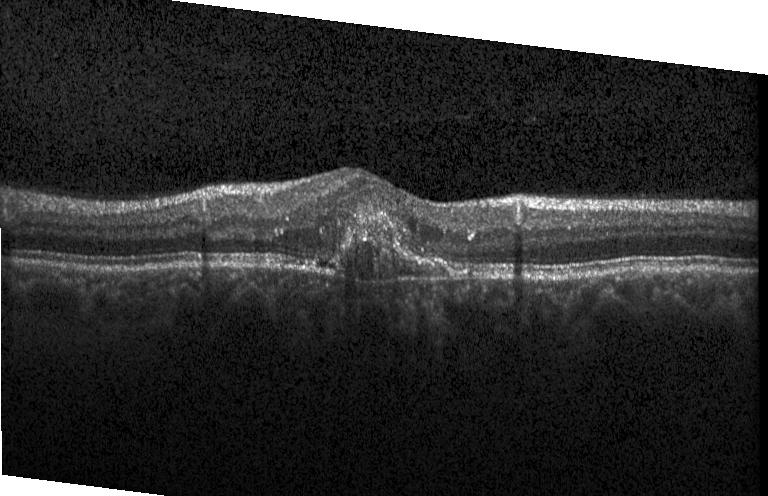

Assessment: a choroidal neovascular membrane.